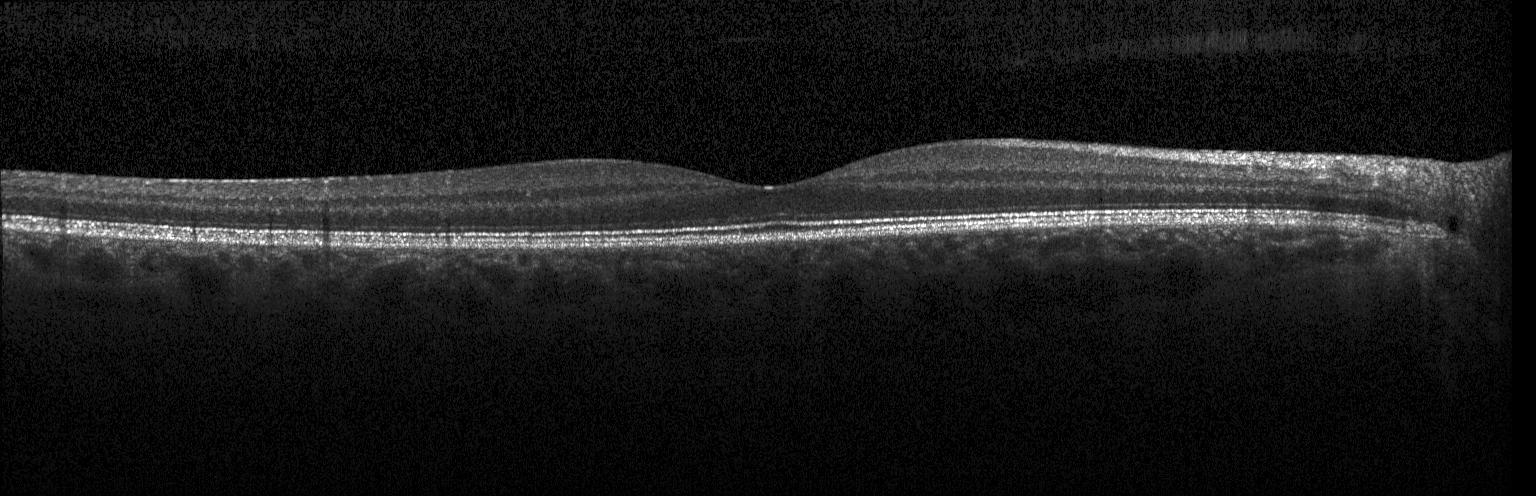

Impression: neither choroidal neovascularization, diabetic macular edema, nor drusen.